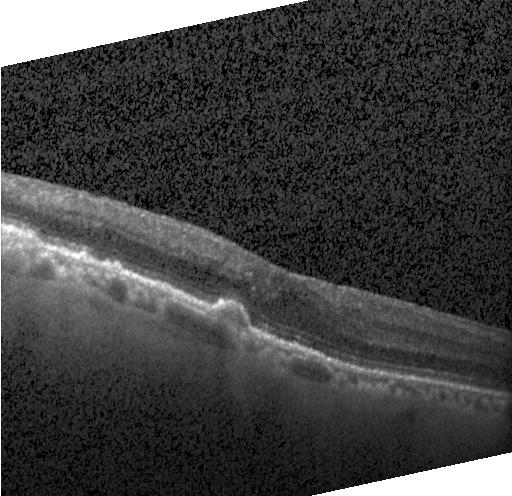
Spectral-domain OCT B-scan: choroidal neovascularization.